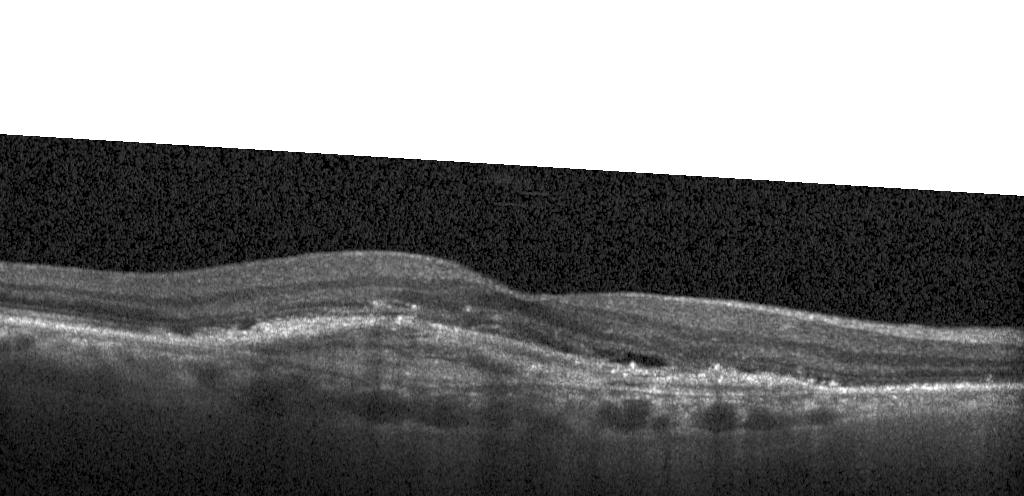 Retinal OCT cross-section
Macular OCT: CNV.